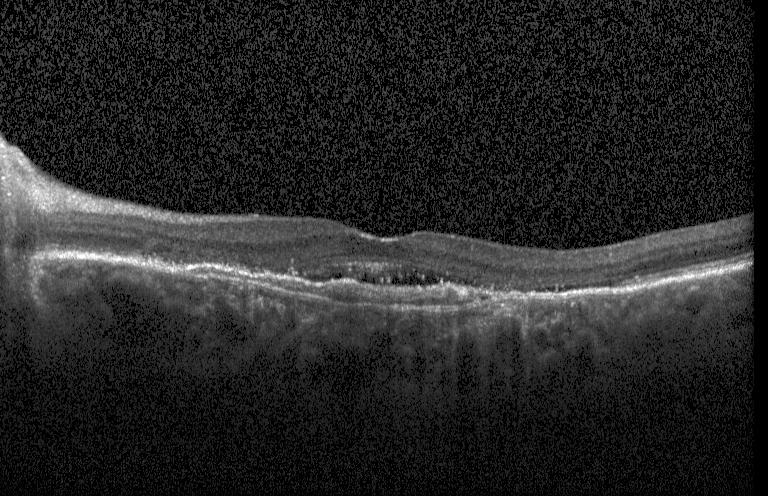

Retinal OCT cross-section
OCT finding: a choroidal neovascular membrane.